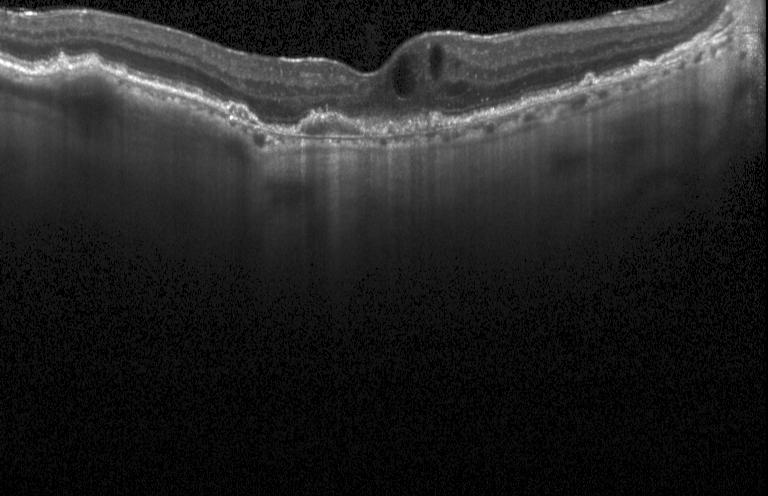 Optical coherence tomography B-scan.
This B-scan demonstrates choroidal neovascularization.